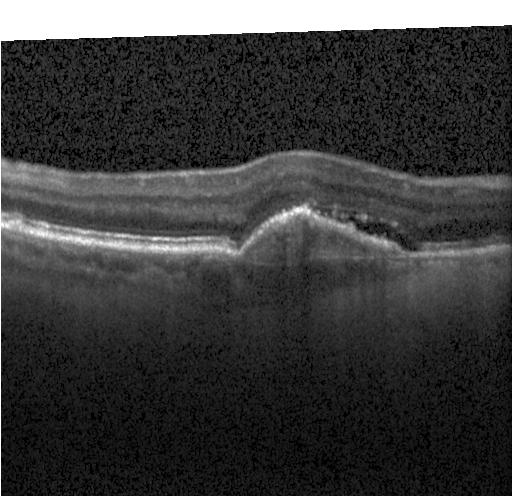

Horizontal scan through the fovea. Retinal OCT B-scan. Spectral-domain optical coherence tomography — Finding: a choroidal neovascular membrane.